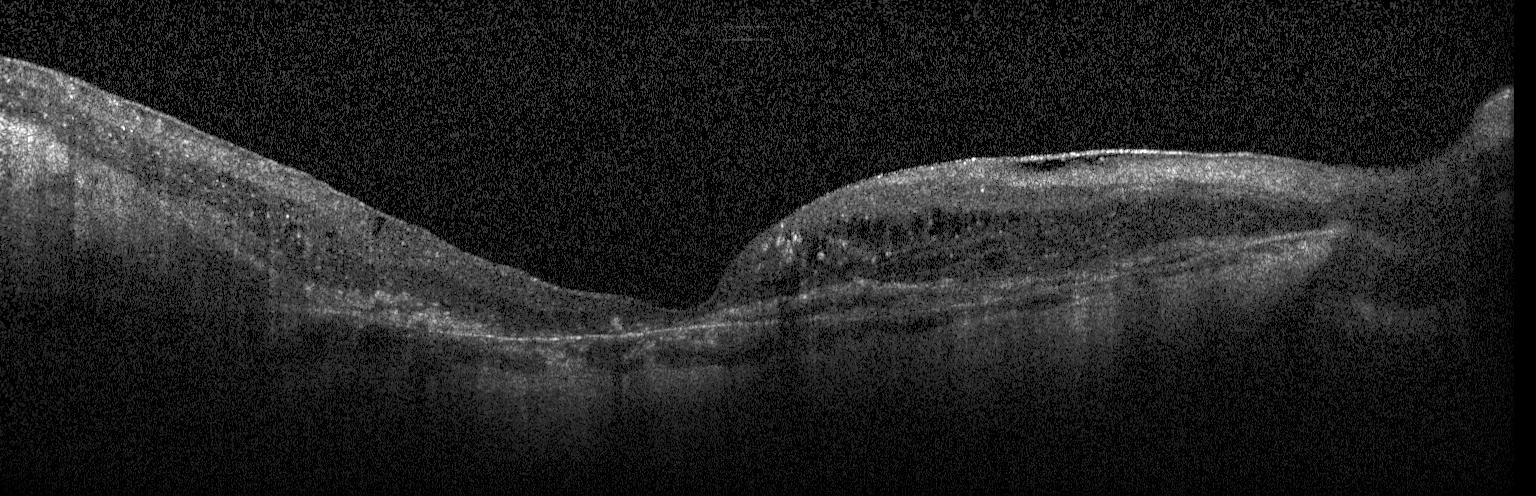 Retinal OCT B-scan
Impression: CNV.